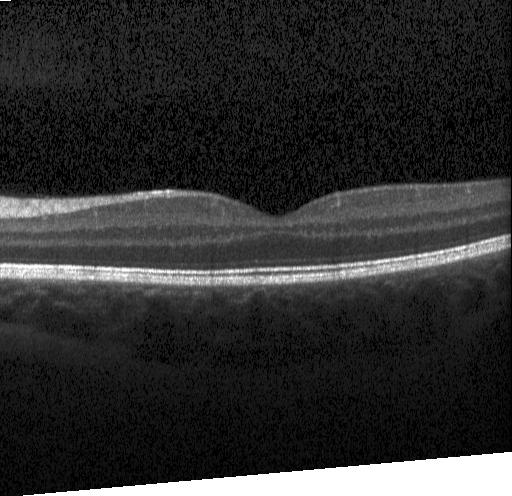
Finding: no evidence of choroidal neovascularization, diabetic macular edema, or drusen.